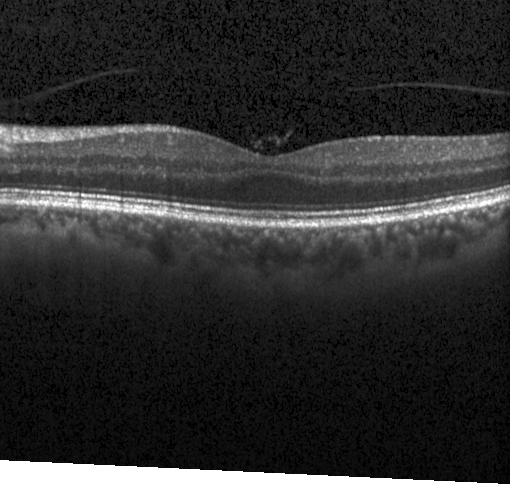 Heidelberg Spectralis. OCT line scan.
This B-scan demonstrates no evidence of choroidal neovascularization, diabetic macular edema, or drusen.